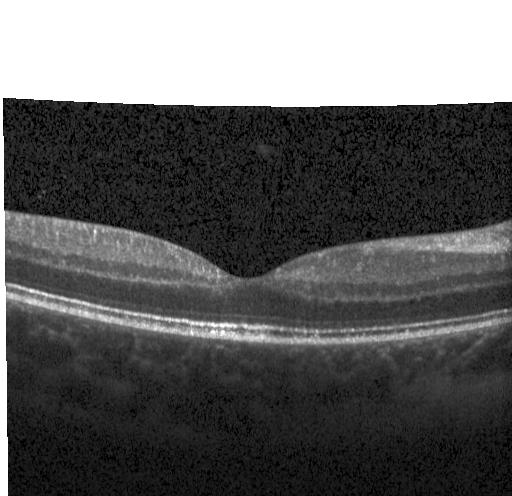

Horizontal scan through the fovea · spectral-domain OCT · retinal OCT B-scan.
OCT finding: no choroidal neovascularization, diabetic macular edema, or drusen.